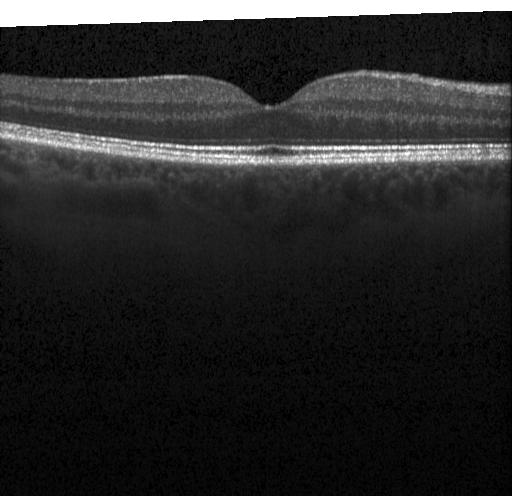

Acquired on a Heidelberg Spectralis; optical coherence tomography B-scan; spectral-domain optical coherence tomography
The scan shows no choroidal neovascularization, diabetic macular edema, or drusen.